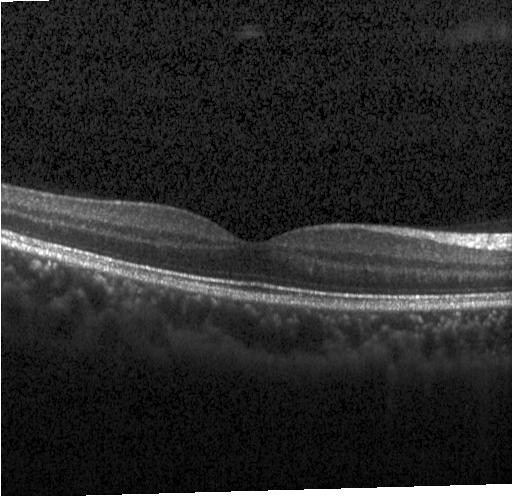

Macular OCT demonstrating no evidence of choroidal neovascularization, diabetic macular edema, or drusen.